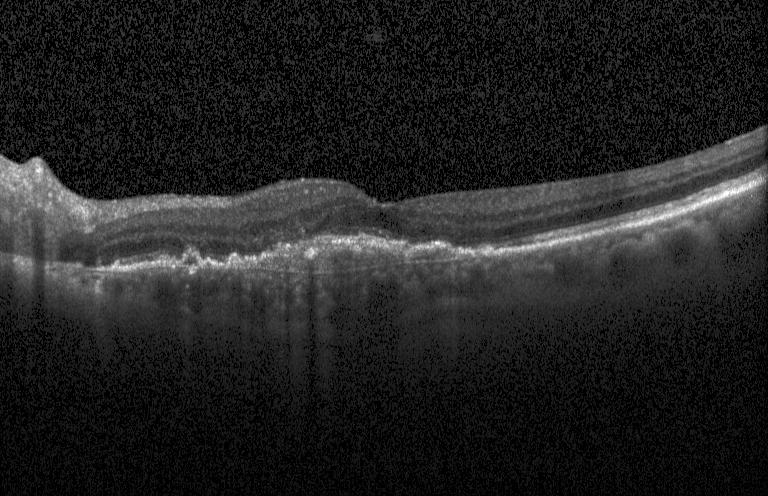 Assessment: a choroidal neovascular membrane.